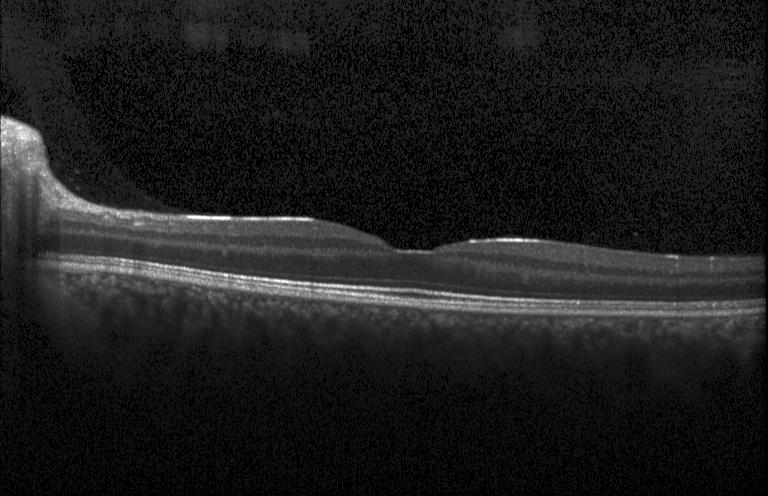

Impression: neither choroidal neovascularization, diabetic macular edema, nor drusen.